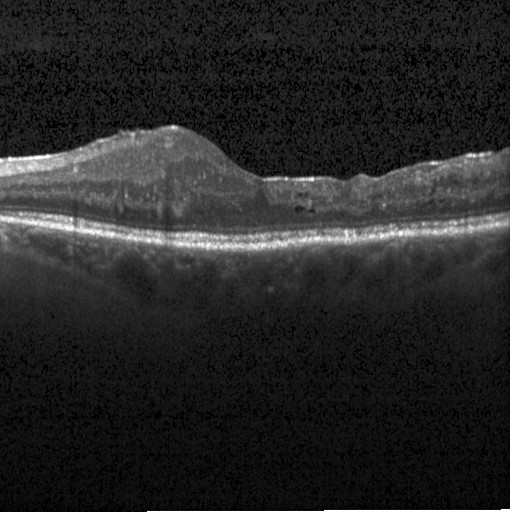 Retinal OCT cross-section, macular scan, spectral-domain OCT — Assessment: diabetic macular edema.